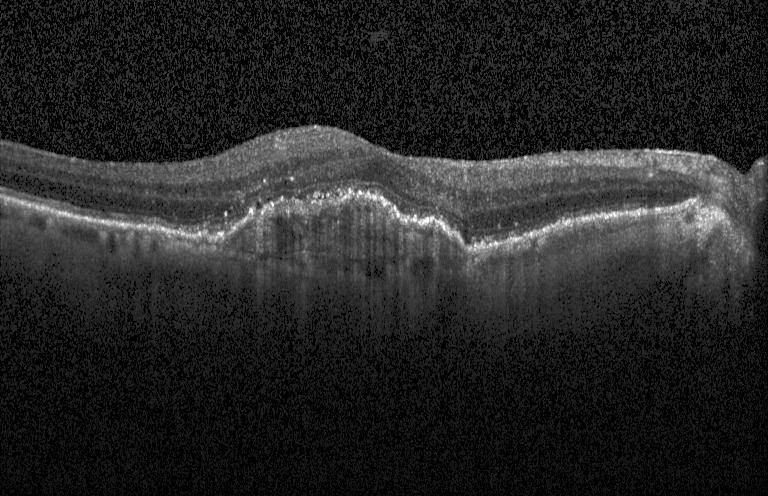 SD-OCT. OCT line scan. Assessment: CNV.